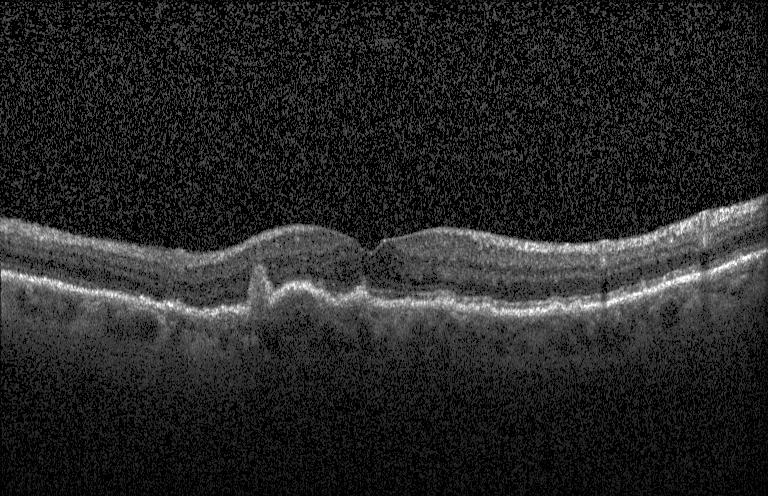
Through the macula. Retinal OCT B-scan — Impression: a choroidal neovascular membrane.